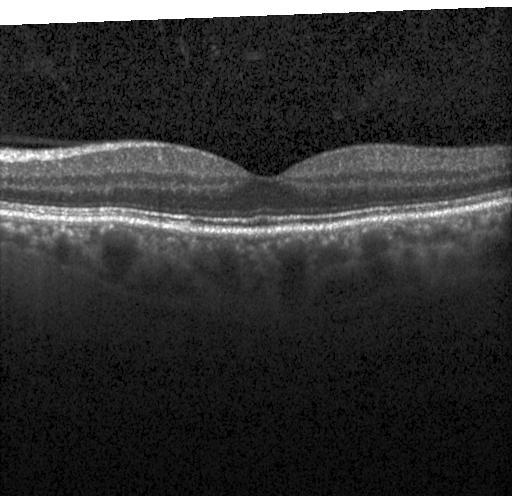
Spectral-domain OCT. Acquired on a Heidelberg Spectralis. Retinal OCT cross-section. Assessment: no choroidal neovascularization, diabetic macular edema, or drusen.